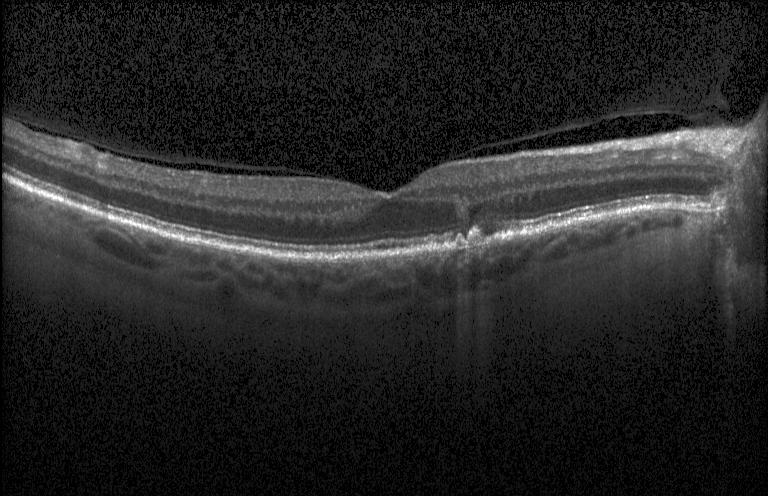

Macular OCT: sub-RPE drusenoid deposits.